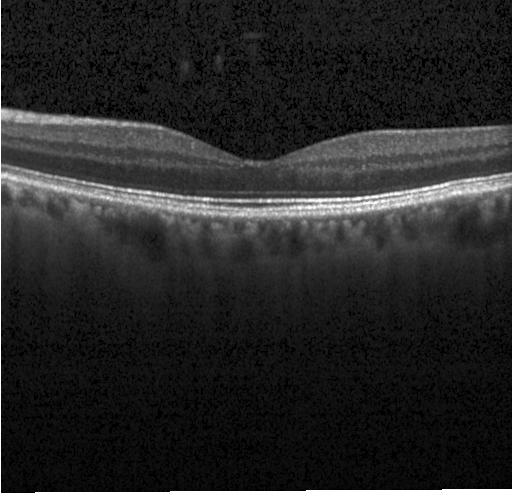

Retinal OCT cross-section. Assessment: no evidence of CNV, DME, or drusen.